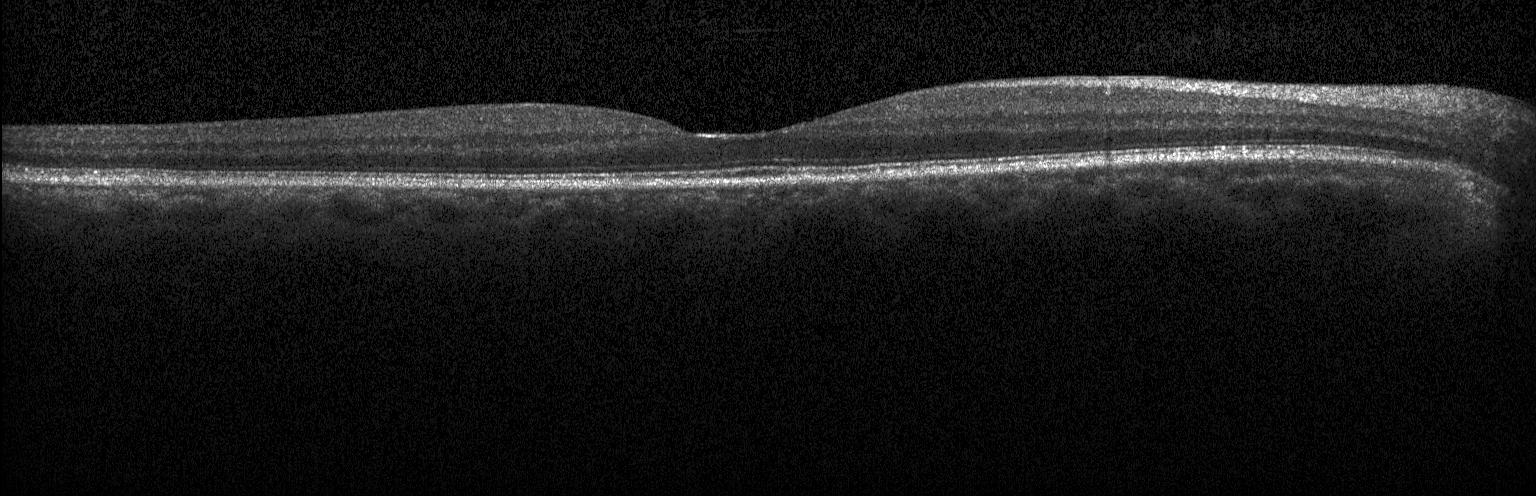 OCT B-scan
Impression: no choroidal neovascularization, no diabetic macular edema, and no drusen.